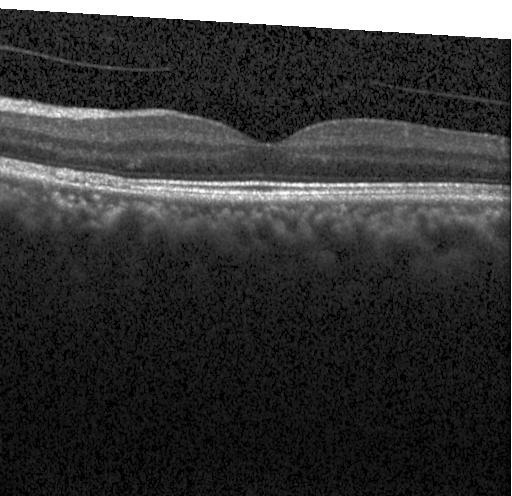
Macular OCT: neither choroidal neovascularization, diabetic macular edema, nor drusen.